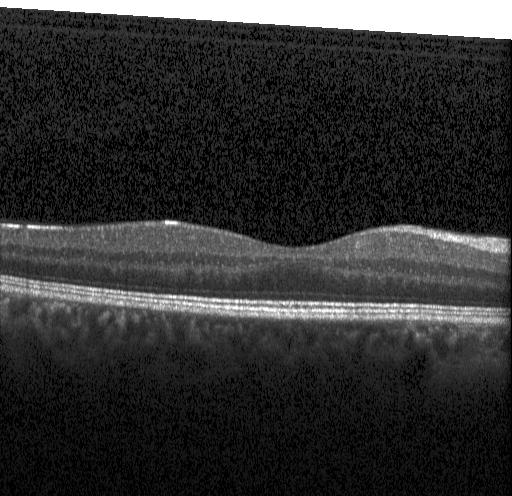 SD-OCT. OCT line scan. Acquired on a Heidelberg Spectralis. Centered on the fovea.
Finding: no CNV, DME, or drusen.